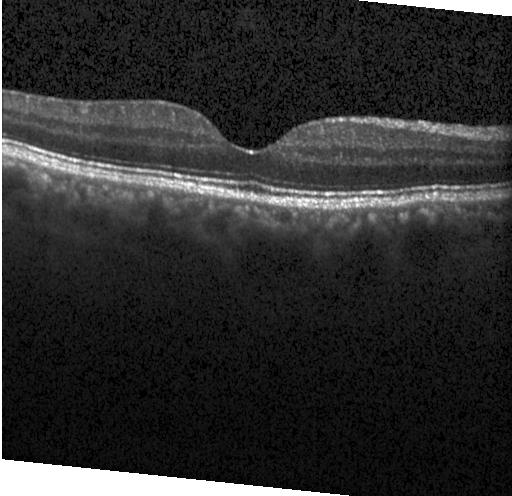 Finding: neither choroidal neovascularization, diabetic macular edema, nor drusen.